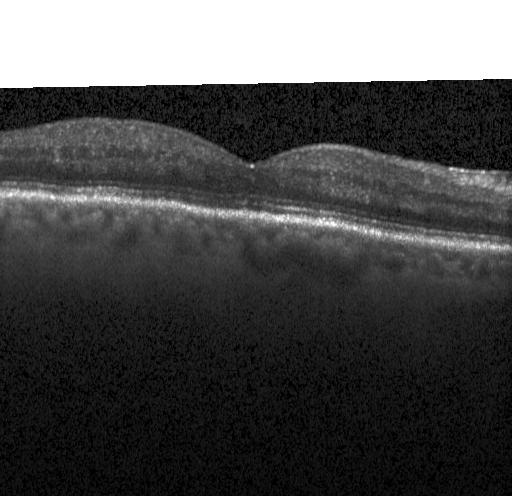
Retinal OCT B-scan, instrument: Heidelberg Spectralis, spectral-domain optical coherence tomography — Diagnosis: no evidence of choroidal neovascularization, diabetic macular edema, or drusen.